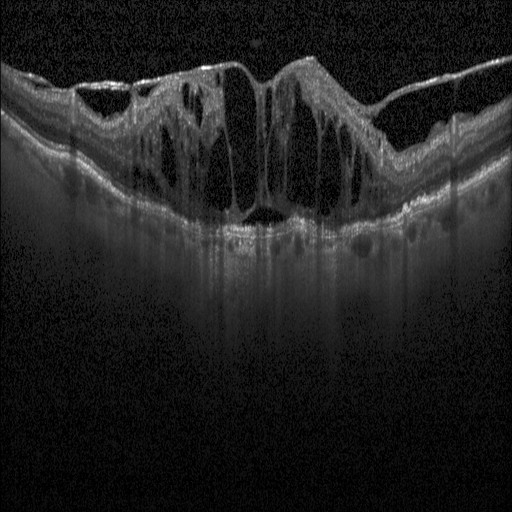 Optical coherence tomography scan
Finding: diabetic macular edema (DME).